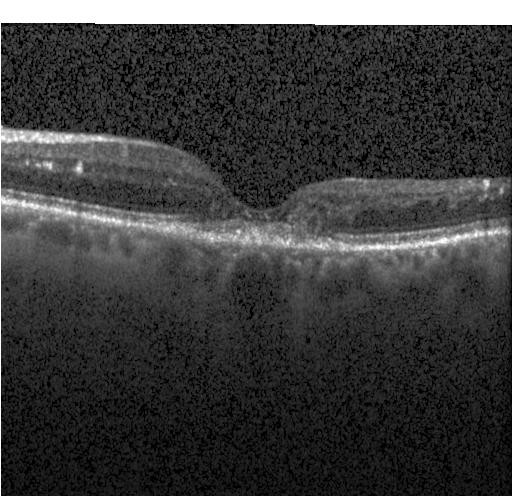

Macular OCT: a choroidal neovascular membrane.